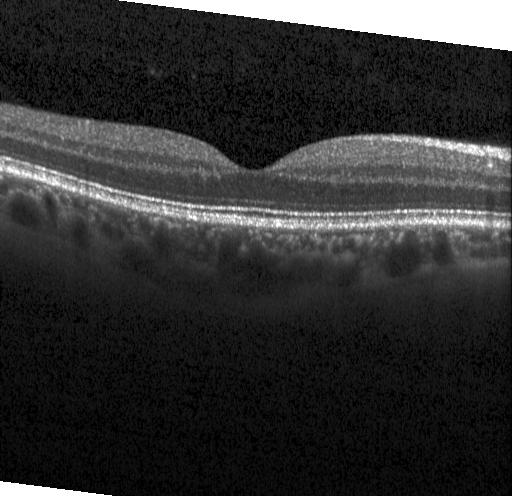

Optical coherence tomography scan · fovea-centered · spectral-domain OCT · Heidelberg Spectralis OCT system. Diagnosis: no choroidal neovascularization, diabetic macular edema, or drusen.